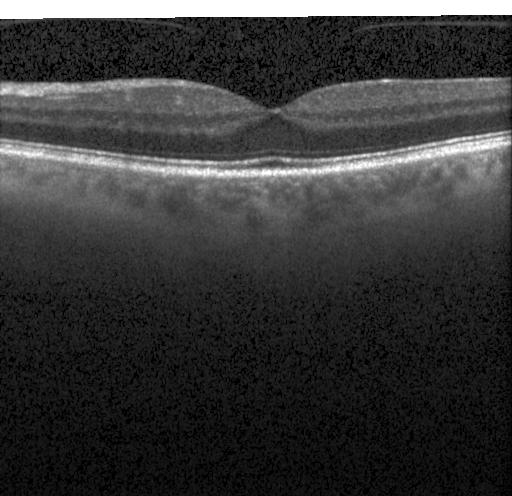

Fovea-centered, optical coherence tomography scan — This B-scan demonstrates no choroidal neovascularization, diabetic macular edema, or drusen.